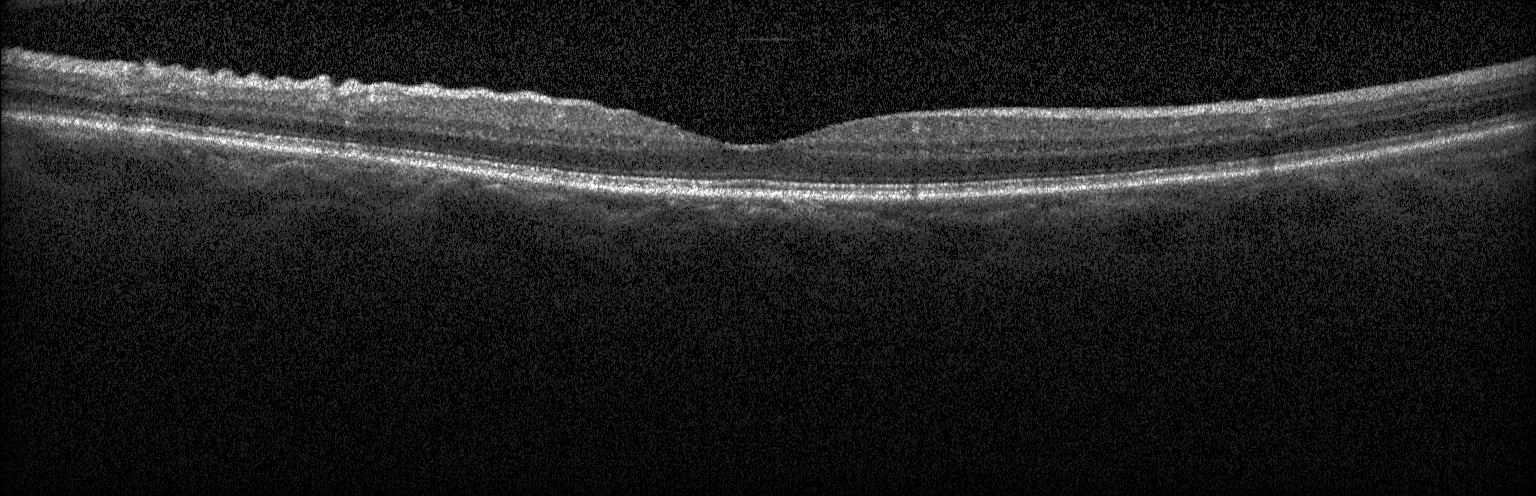
Assessment: no choroidal neovascularization, diabetic macular edema, or drusen.